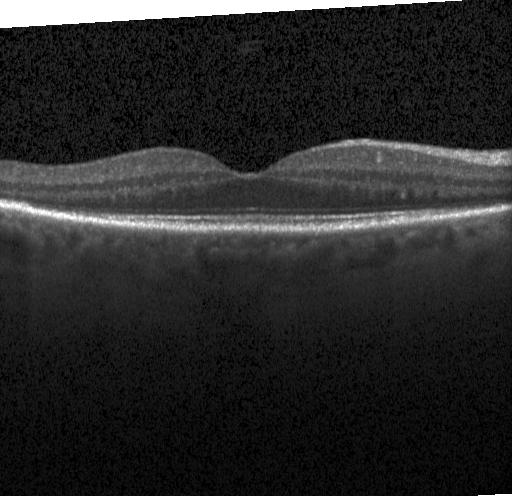

Spectral-domain OCT; OCT B-scan; instrument: Heidelberg Spectralis
Diagnosis: no choroidal neovascularization, diabetic macular edema, or drusen.